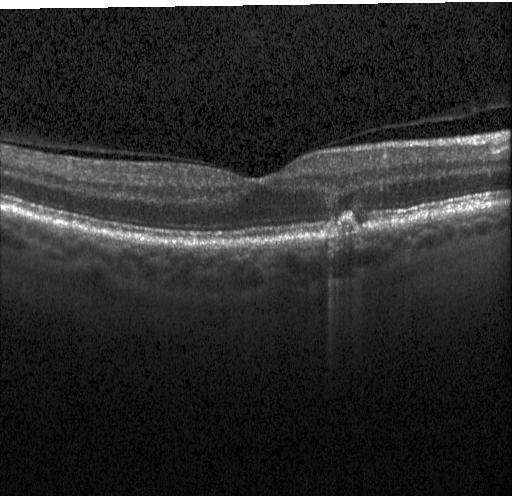
Dx: sub-RPE drusenoid deposits.